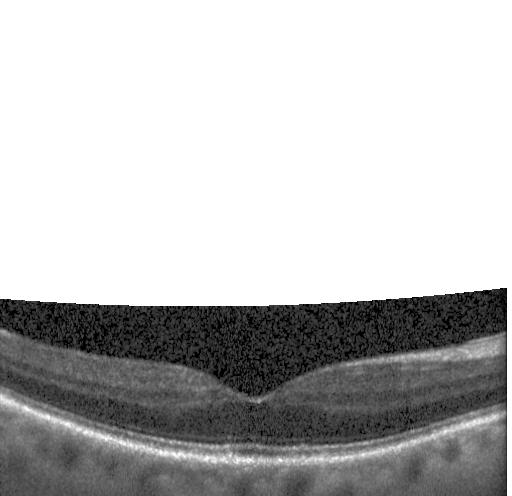 Retinal OCT cross-section. Horizontal scan through the fovea. Spectral-domain OCT
Dx: no choroidal neovascularization, diabetic macular edema, or drusen.